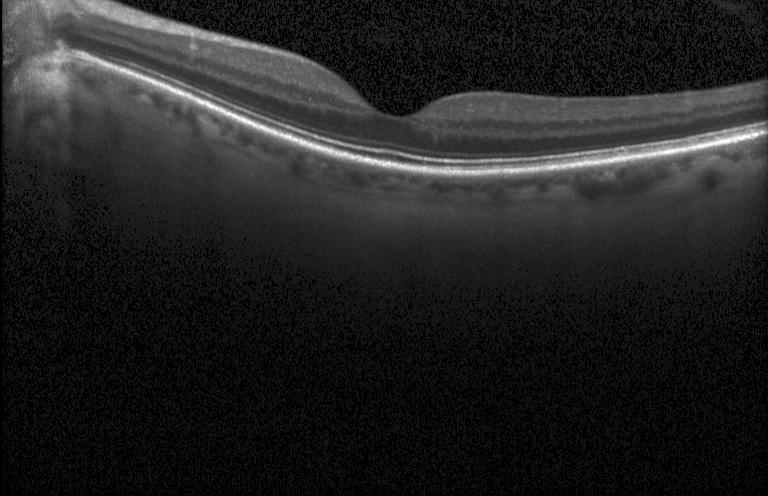

OCT scan showing no choroidal neovascularization, diabetic macular edema, or drusen.